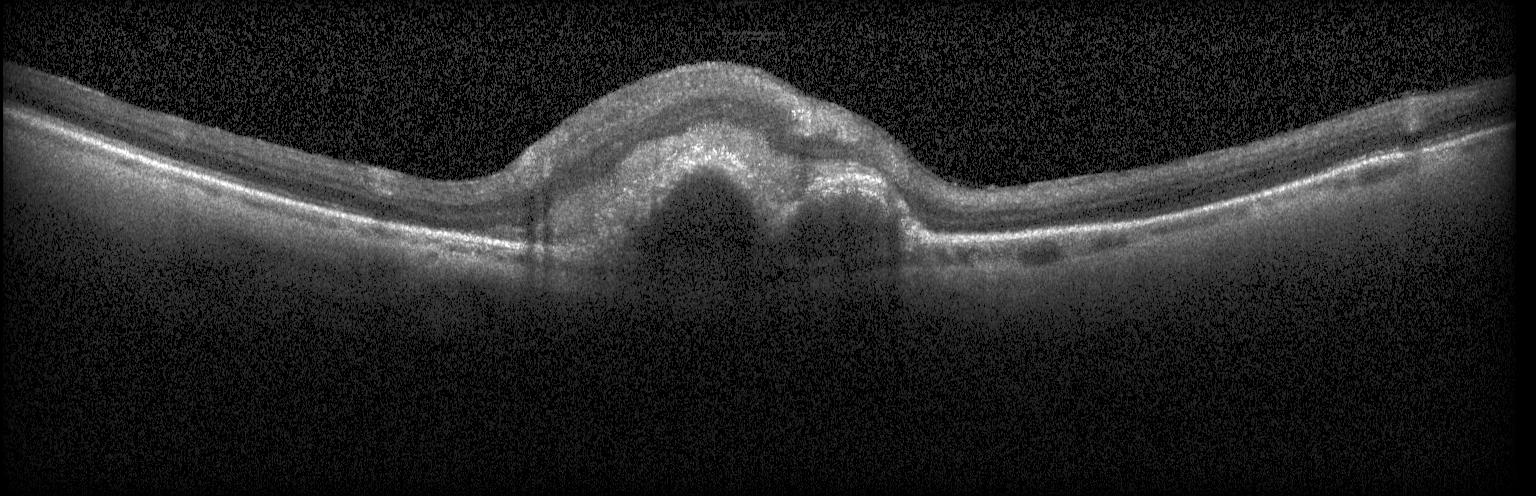
Horizontal scan through the fovea. Retinal OCT B-scan
Choroidal neovascularization (CNV).